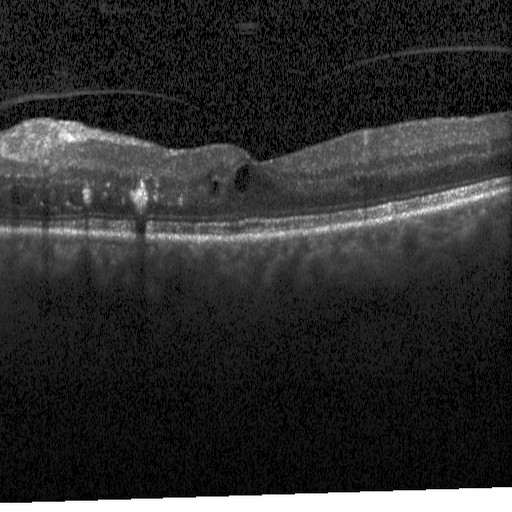 Finding: diabetic macular edema (DME).